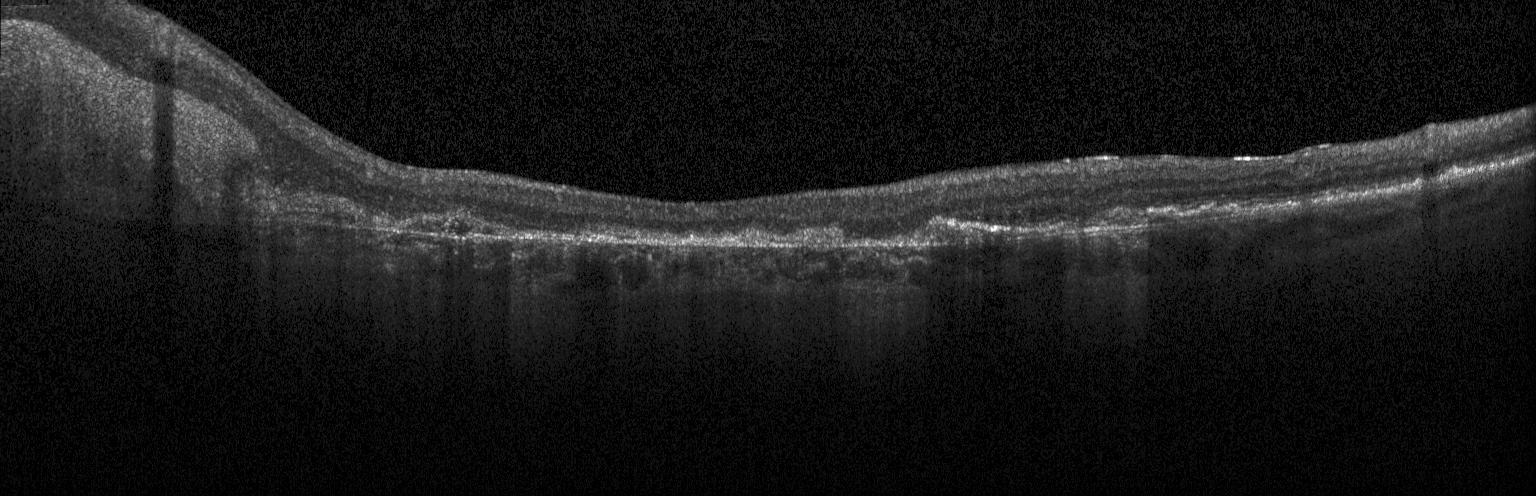
Optical coherence tomography scan; through the macula; SD-OCT; acquired on a Heidelberg Spectralis
This B-scan demonstrates choroidal neovascularization.